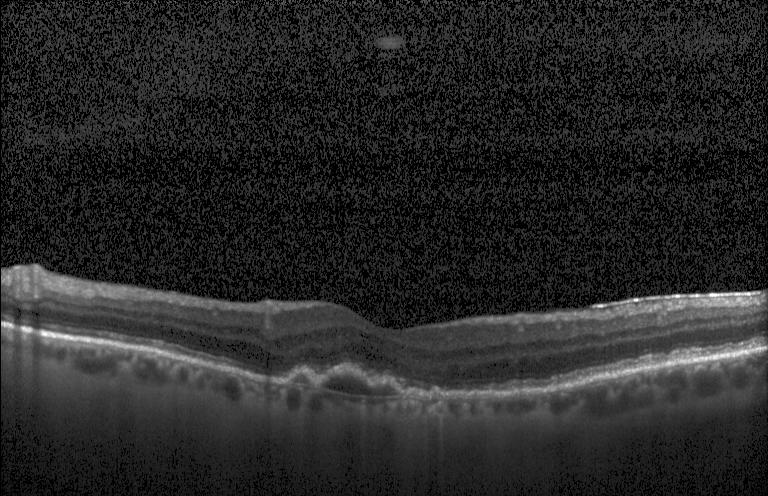
Finding: a choroidal neovascular membrane.